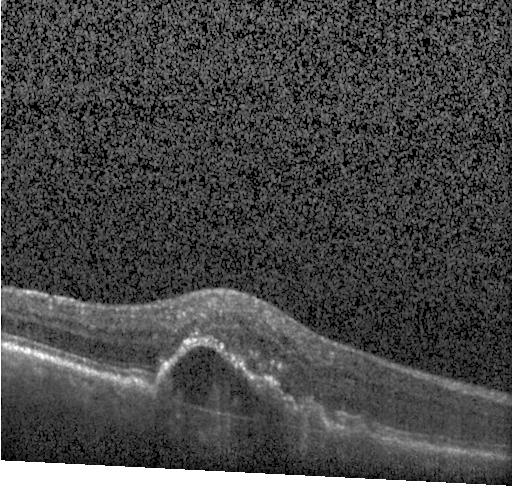

Instrument: Heidelberg Spectralis · through the macula · retinal OCT B-scan — Finding: a choroidal neovascular membrane.